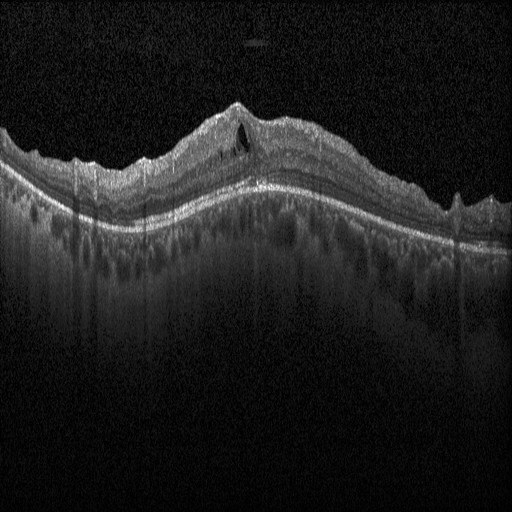
Spectral-domain OCT · retinal OCT cross-section · horizontal scan through the fovea
The scan shows diabetic macular edema (DME).